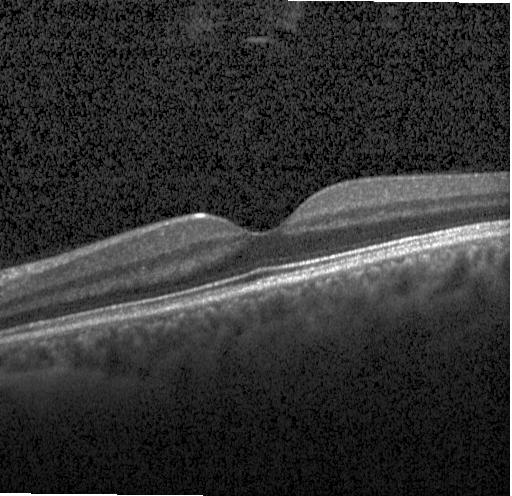 Optical coherence tomography B-scan. Fovea-centered. Spectral-domain OCT
Neither CNV, DME, nor drusen.